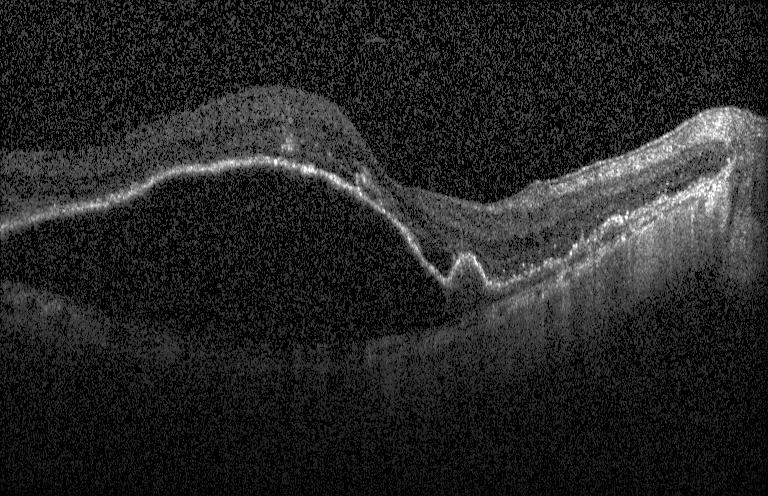
Retinal OCT B-scan. Diagnosis: choroidal neovascularization.